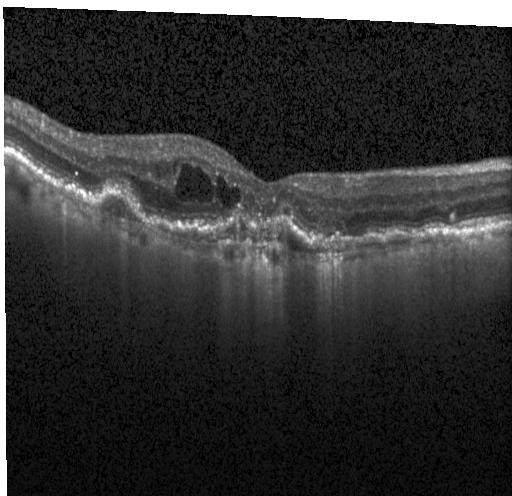 Macular scan · OCT line scan · spectral-domain optical coherence tomography · instrument: Heidelberg Spectralis
Diagnosis: CNV.